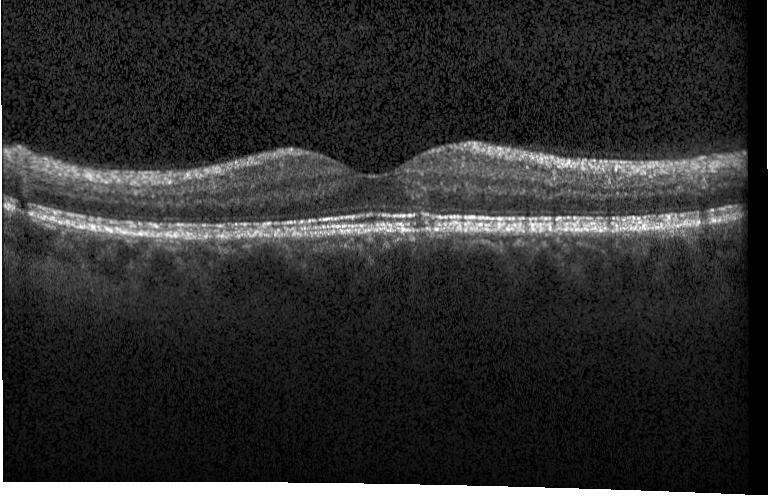

OCT scan showing neither CNV, DME, nor drusen.